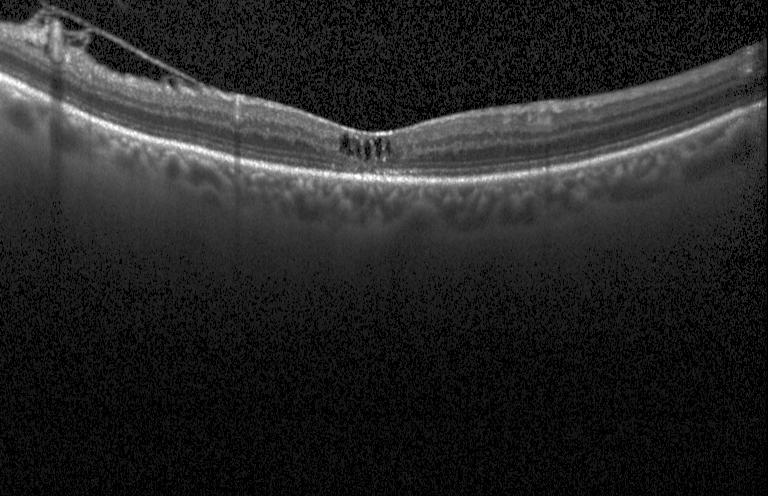 Macular OCT: DME.